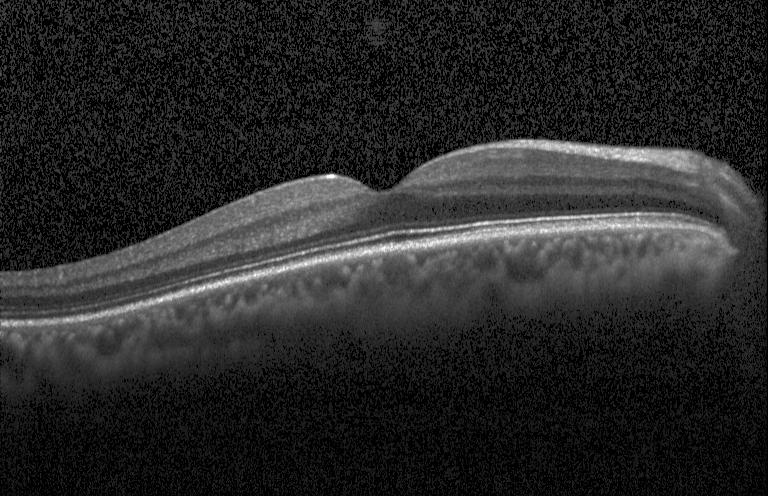

Spectral-domain OCT, retinal OCT B-scan, Heidelberg Spectralis.
Finding: no evidence of choroidal neovascularization, diabetic macular edema, or drusen.